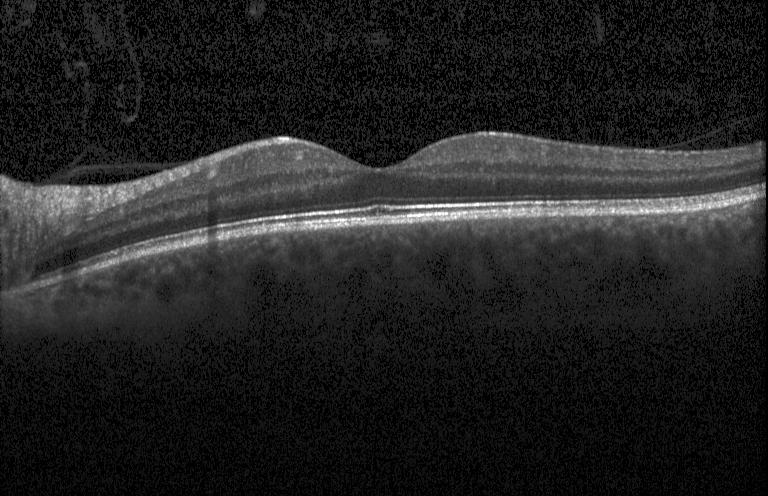 OCT line scan — Impression: no CNV, DME, or drusen.